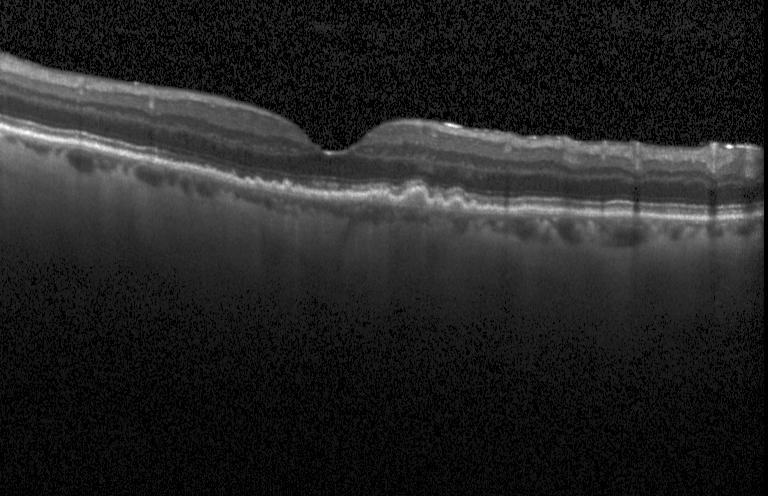
Optical coherence tomography B-scan — Diagnosis: sub-RPE drusenoid deposits.